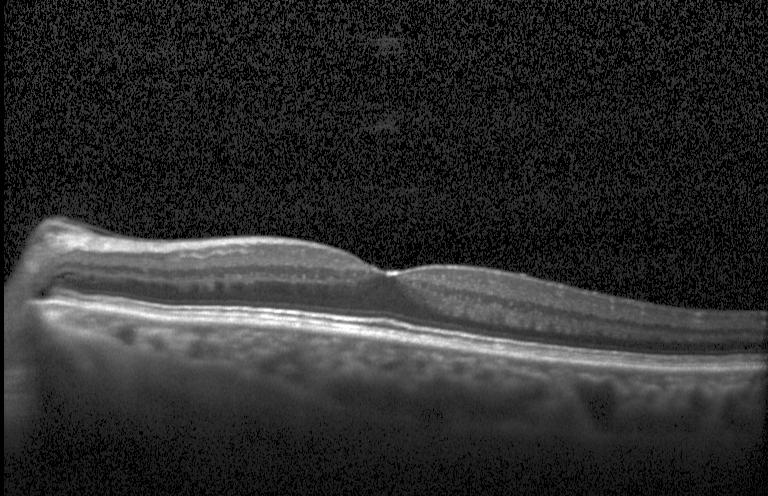
Optical coherence tomography B-scan; fovea-centered
Impression: neither choroidal neovascularization, diabetic macular edema, nor drusen.